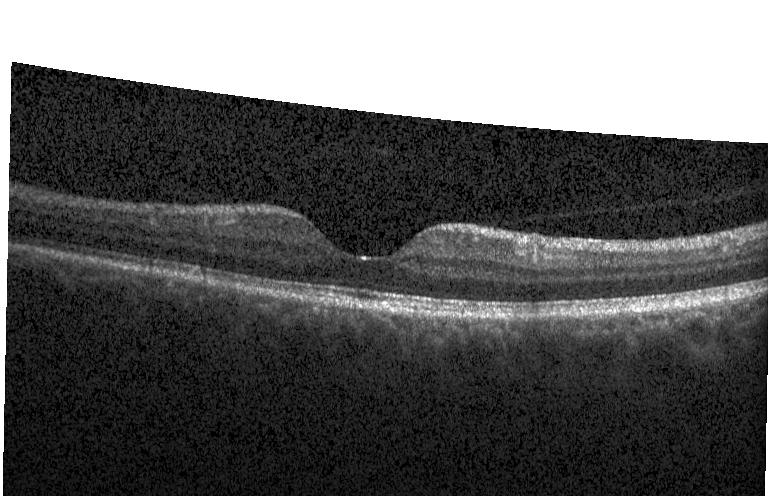

Diagnosis: no evidence of CNV, DME, or drusen.